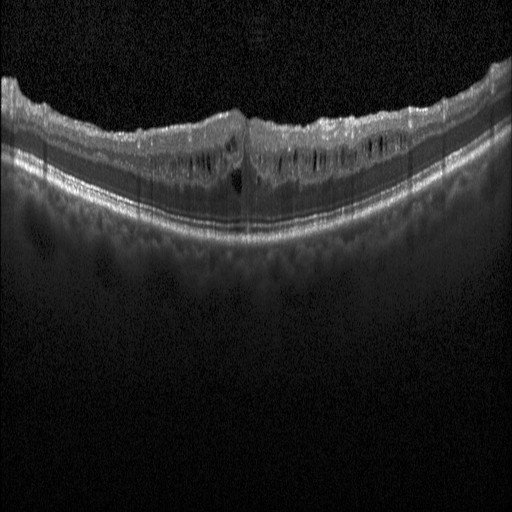

Diagnosis: DME.